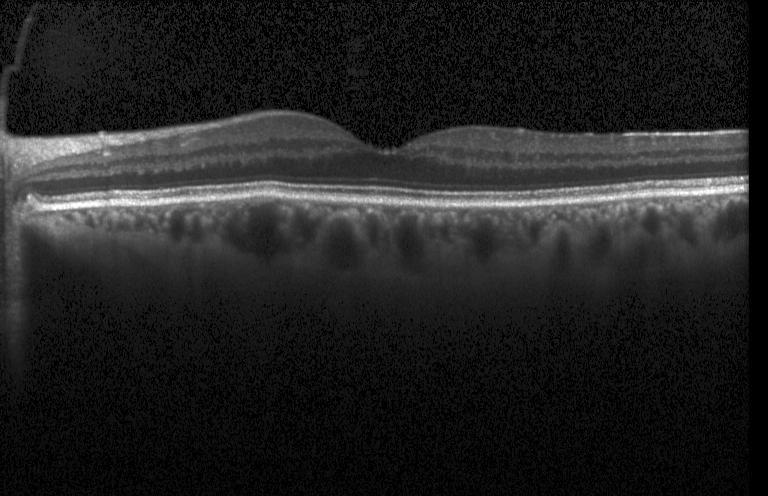
Finding: no choroidal neovascularization, no diabetic macular edema, and no drusen.